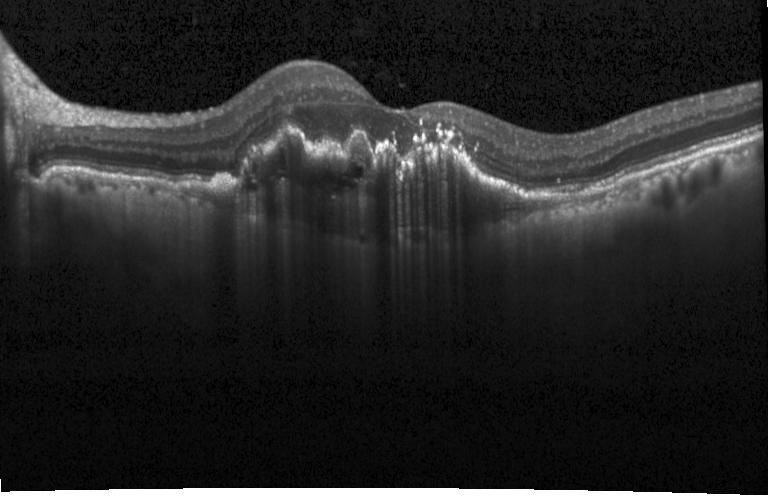

Retinal OCT cross-section showing a choroidal neovascular membrane.